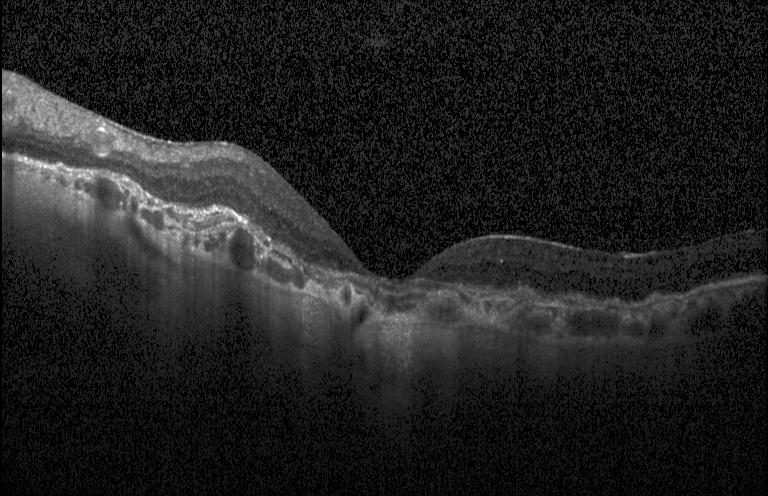
Acquired on a Heidelberg Spectralis · fovea-centered · optical coherence tomography scan · spectral-domain OCT
Finding: CNV.